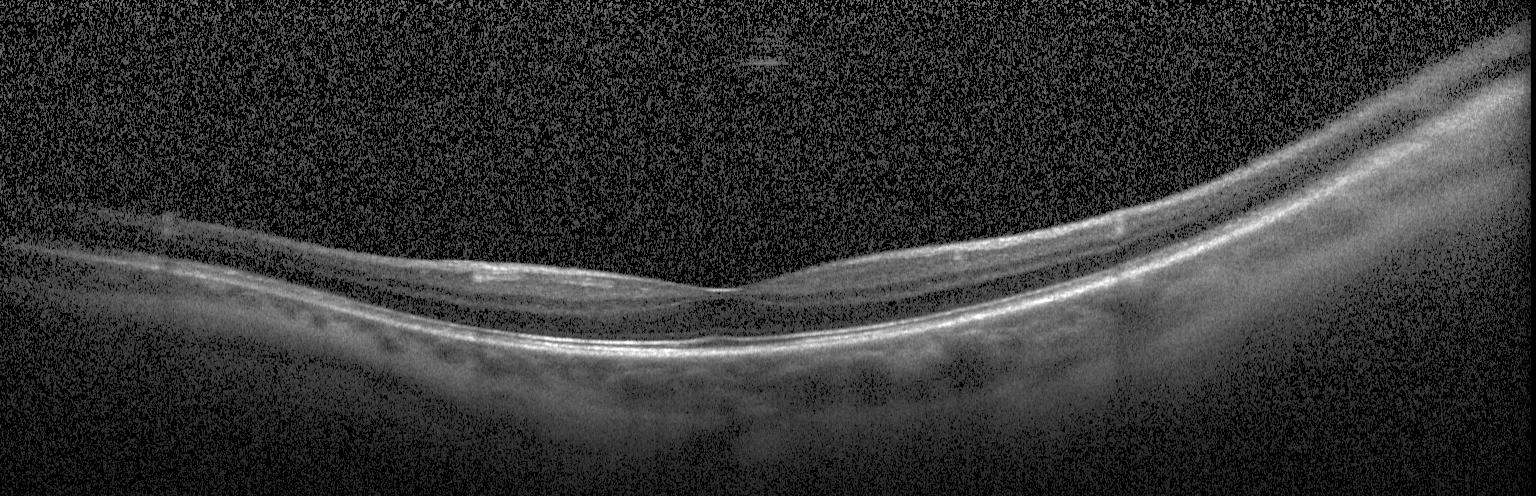

SD-OCT, acquired on a Heidelberg Spectralis, OCT B-scan — This B-scan demonstrates no evidence of choroidal neovascularization, diabetic macular edema, or drusen.